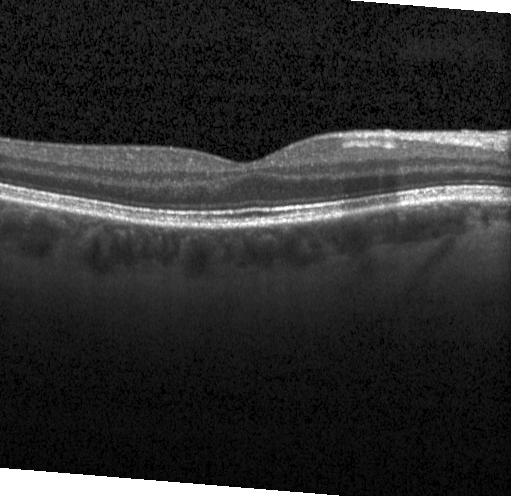
Instrument: Heidelberg Spectralis, SD-OCT, OCT line scan, through the macula
Impression: no choroidal neovascularization, no diabetic macular edema, and no drusen.